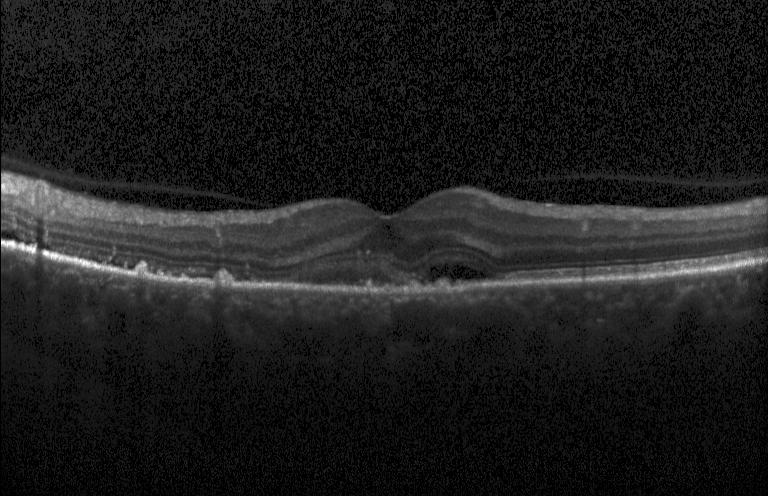

Optical coherence tomography scan · fovea-centered · SD-OCT · Heidelberg Spectralis OCT system — This B-scan demonstrates a choroidal neovascular membrane.